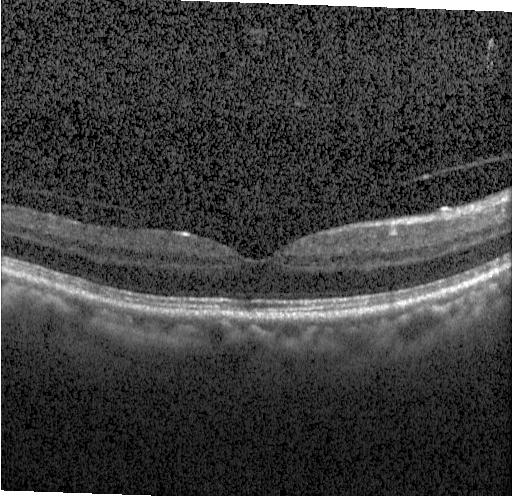 Instrument: Heidelberg Spectralis; spectral-domain OCT; retinal OCT B-scan; centered on the fovea — Impression: no choroidal neovascularization, no diabetic macular edema, and no drusen.